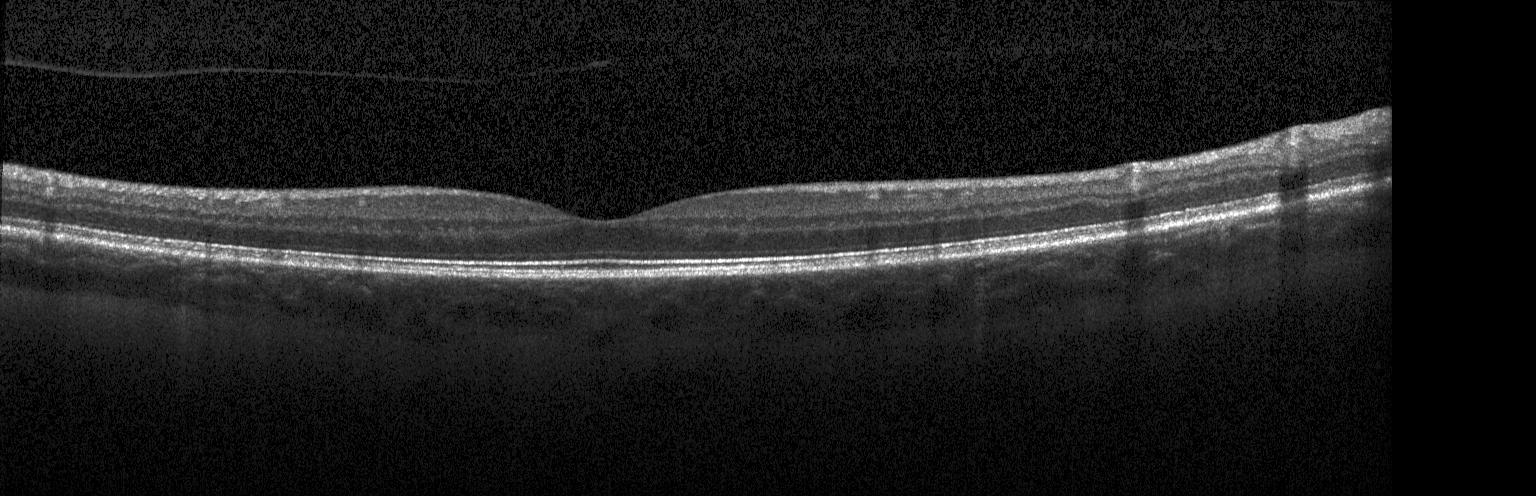

Retinal OCT cross-section. Heidelberg Spectralis OCT system.
Diagnosis: no choroidal neovascularization, no diabetic macular edema, and no drusen.